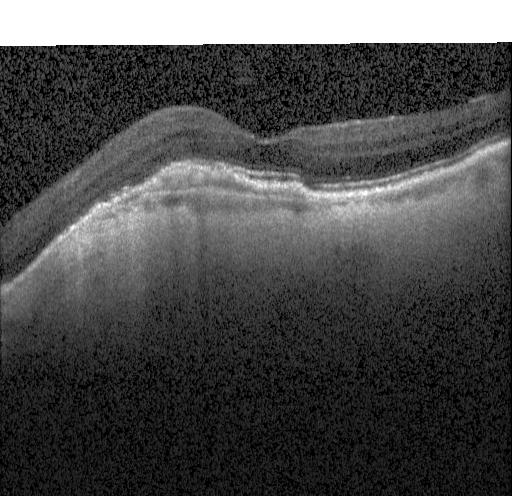
Retinal OCT cross-section · macular scan.
Finding: choroidal neovascularization (CNV).